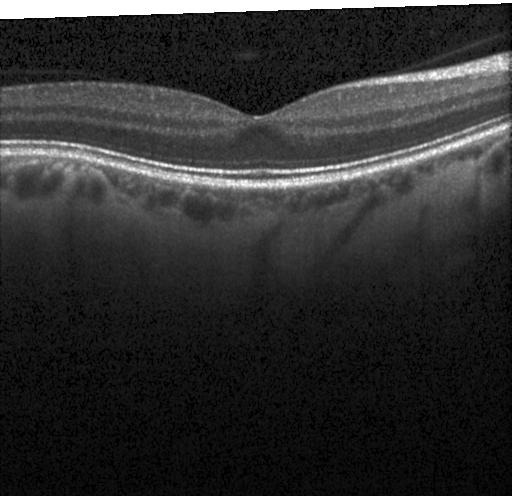
Impression: no choroidal neovascularization, no diabetic macular edema, and no drusen.